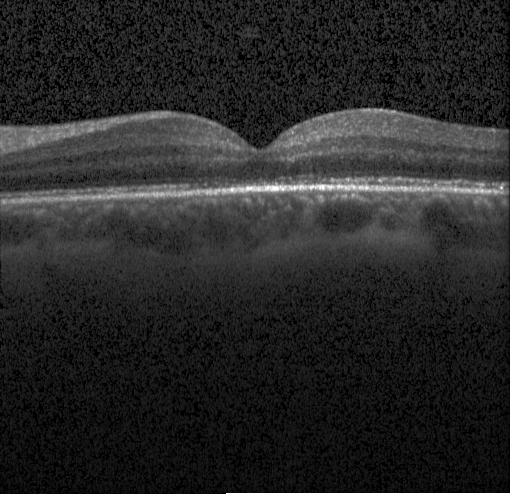
Spectral-domain OCT. Retinal OCT B-scan. Fovea-centered. Heidelberg Spectralis OCT system. Finding: no choroidal neovascularization, no diabetic macular edema, and no drusen.